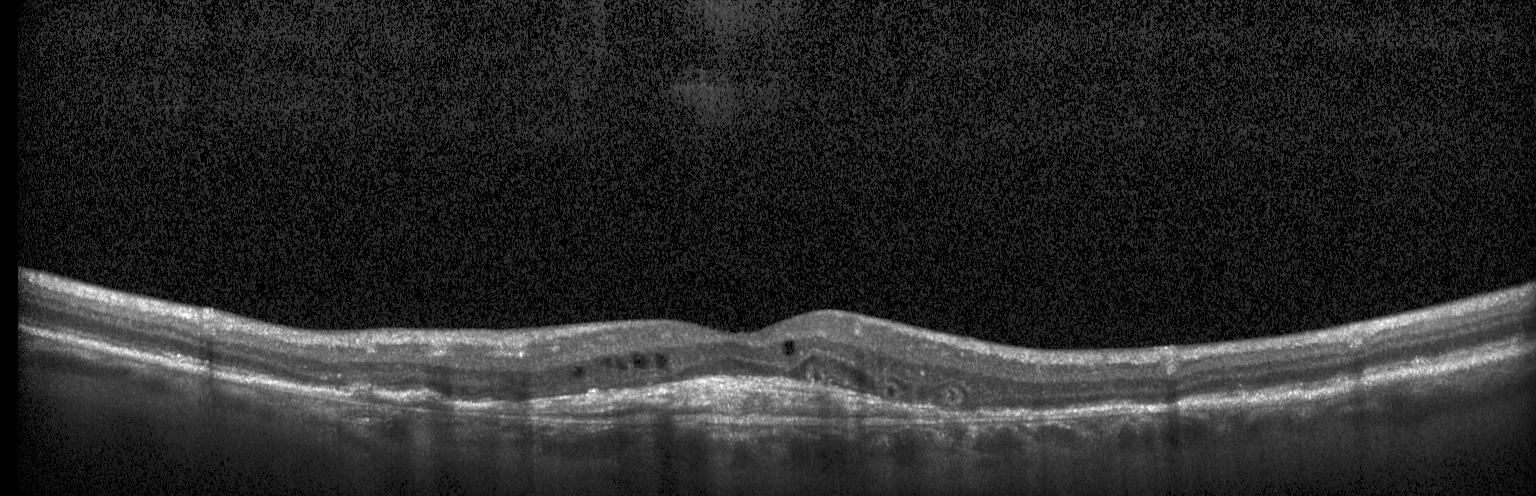 Finding: CNV.